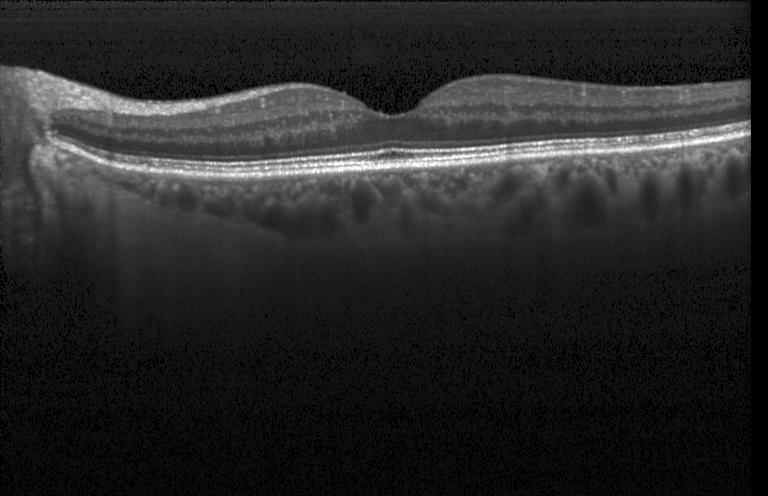
Spectral-domain optical coherence tomography; optical coherence tomography B-scan; through the macula.
Diagnosis: no evidence of CNV, DME, or drusen.